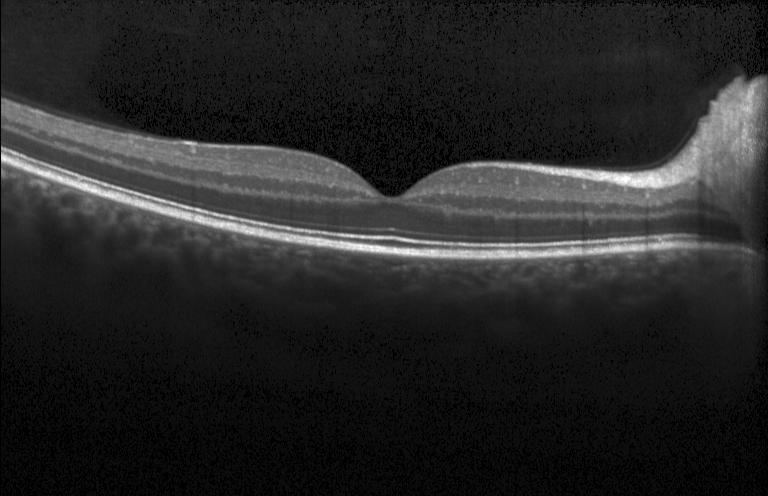

OCT B-scan.
Diagnosis: no CNV, no DME, and no drusen.